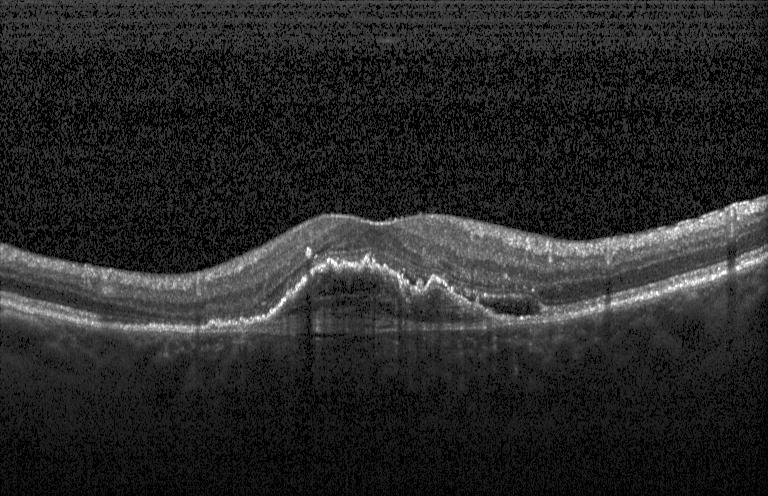
The scan shows a choroidal neovascular membrane.